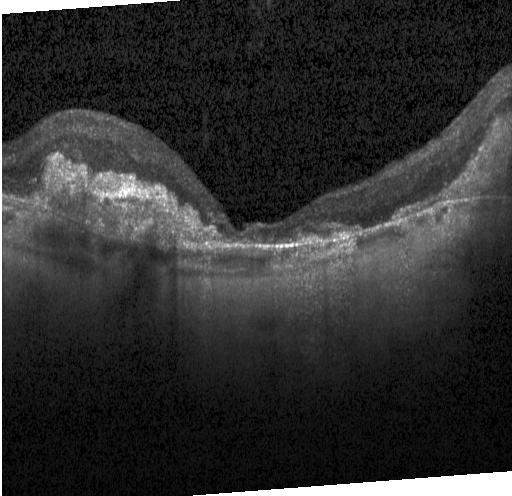

Macular OCT: a choroidal neovascular membrane.